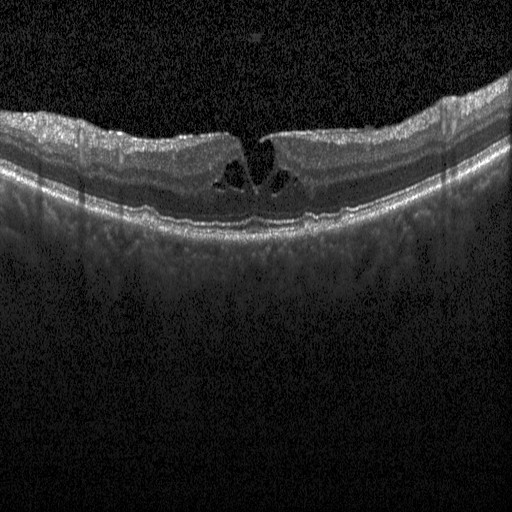

Macular OCT: diabetic macular edema.